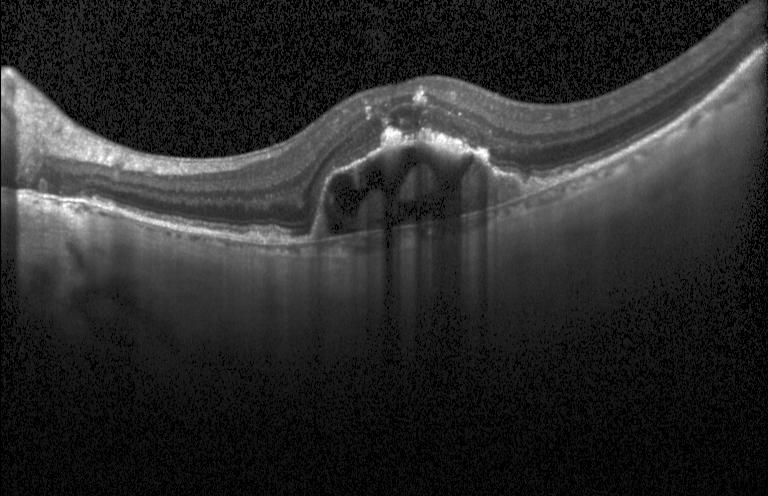

Finding: a choroidal neovascular membrane.